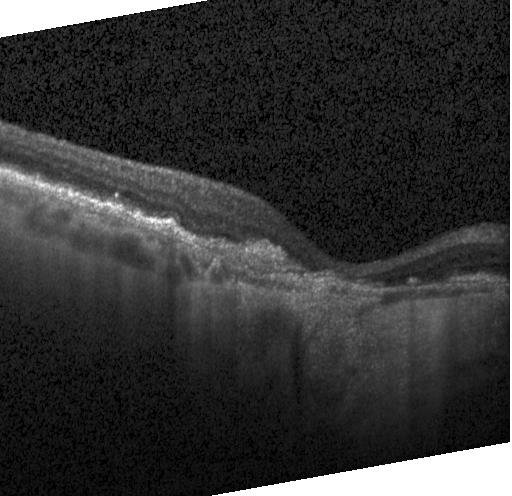
Spectral-domain OCT · centered on the fovea · OCT B-scan — Macular OCT: choroidal neovascularization.